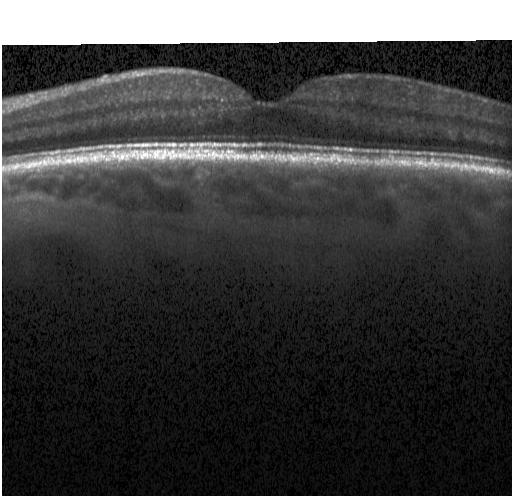 SD-OCT · retinal OCT cross-section · horizontal scan through the fovea · Heidelberg Spectralis OCT system — Impression: no choroidal neovascularization, no diabetic macular edema, and no drusen.